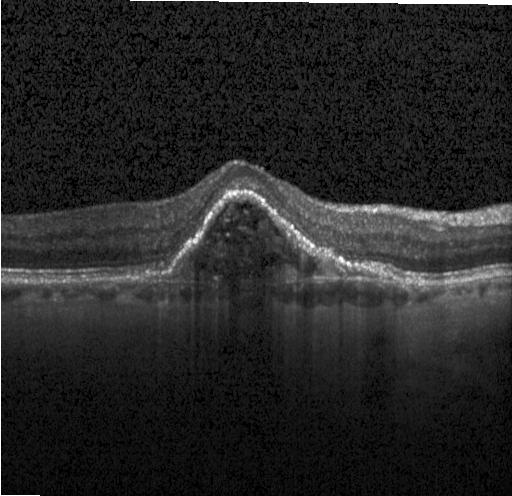 Optical coherence tomography B-scan; Heidelberg Spectralis; through the macula; SD-OCT
Finding: choroidal neovascularization.